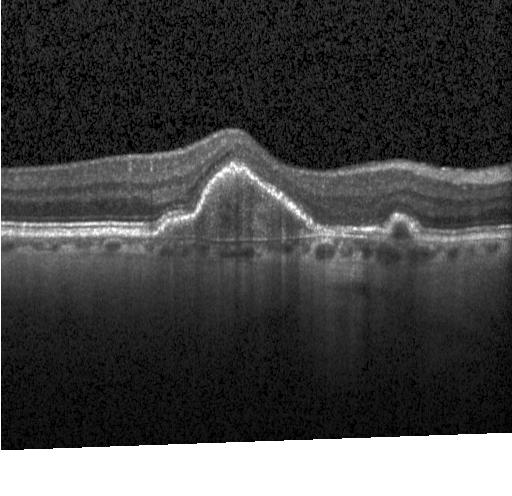 Retinal OCT cross-section showing choroidal neovascularization (CNV).